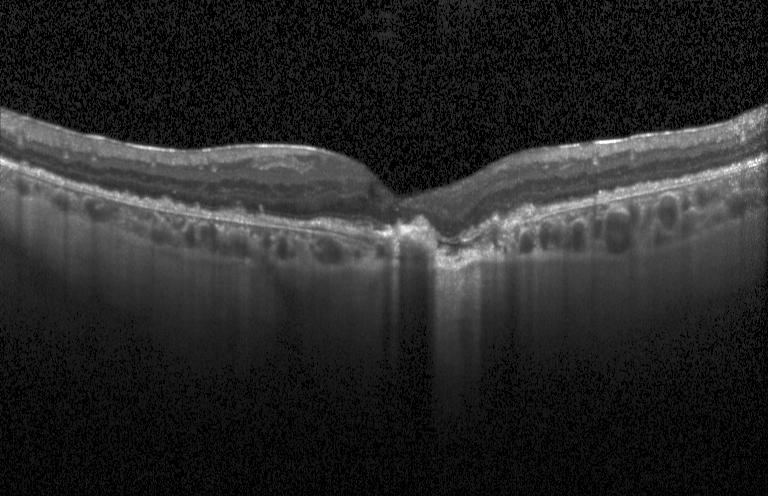

Acquired on a Heidelberg Spectralis. SD-OCT. Optical coherence tomography B-scan.
CNV.